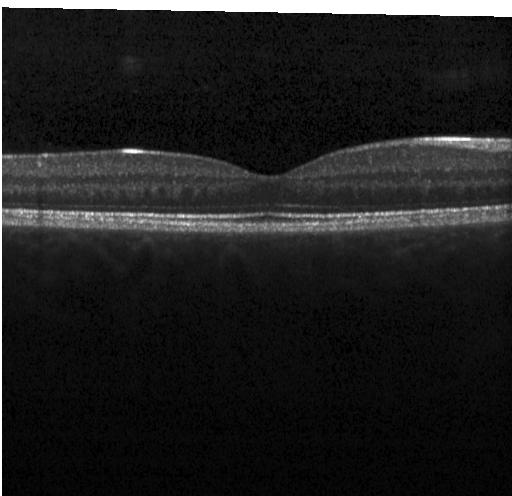

Macular scan; optical coherence tomography scan; spectral-domain OCT. Dx: no choroidal neovascularization, diabetic macular edema, or drusen.